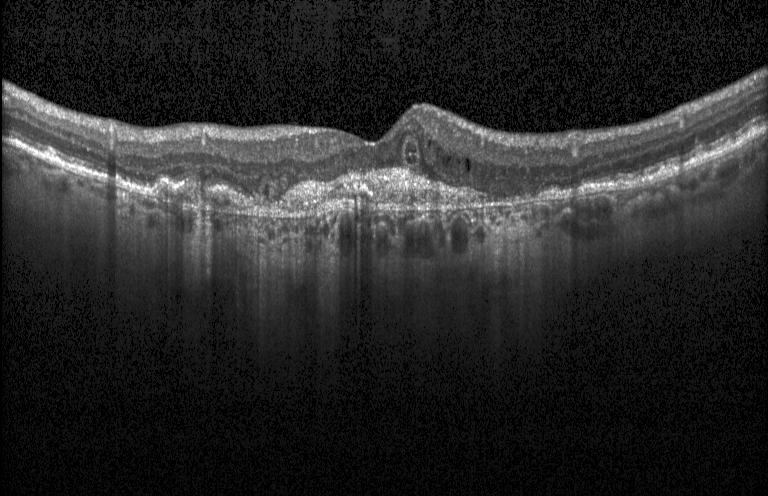
Fovea-centered · retinal OCT cross-section.
Macular OCT: a choroidal neovascular membrane.